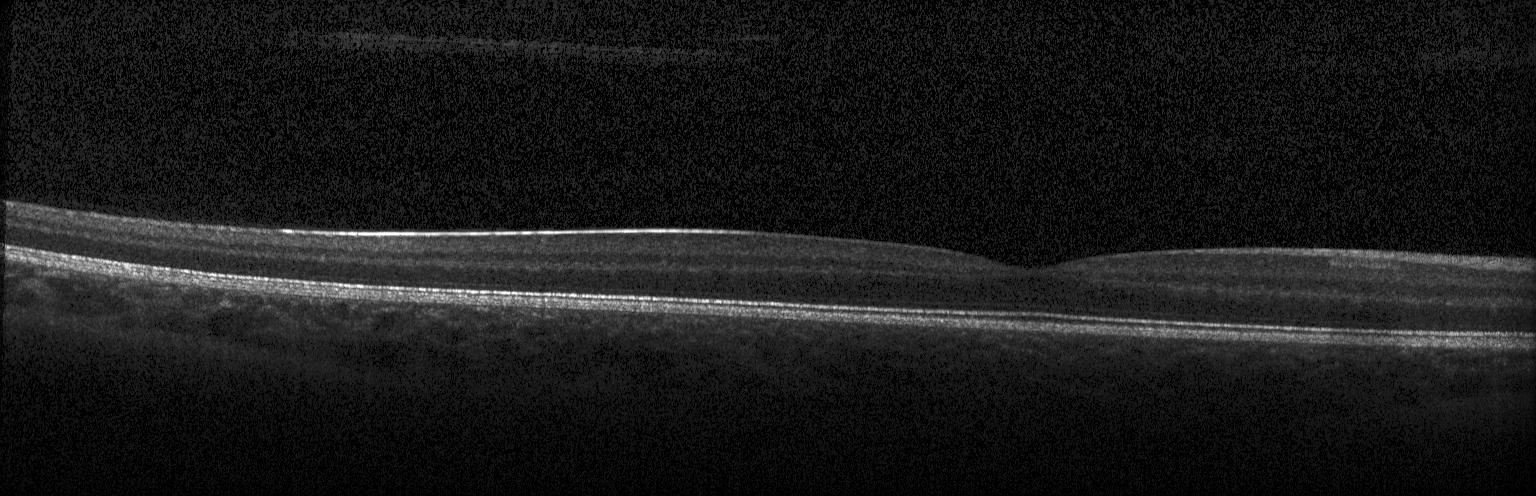 Finding: no CNV, no DME, and no drusen.